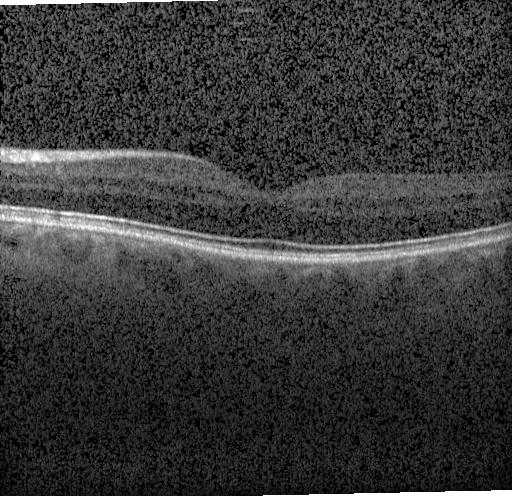

OCT line scan; instrument: Heidelberg Spectralis.
Impression: no CNV, no DME, and no drusen.